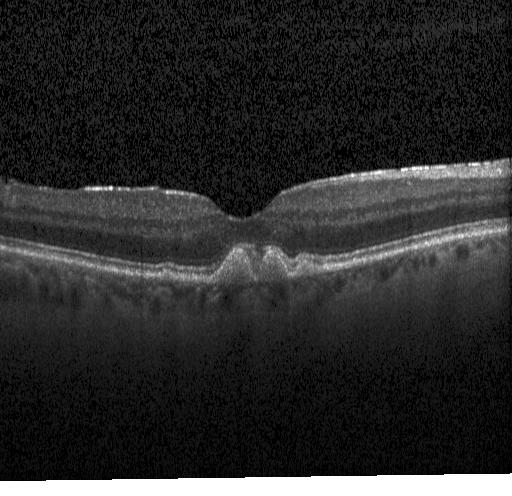

Optical coherence tomography B-scan.
Finding: sub-RPE drusenoid deposits.